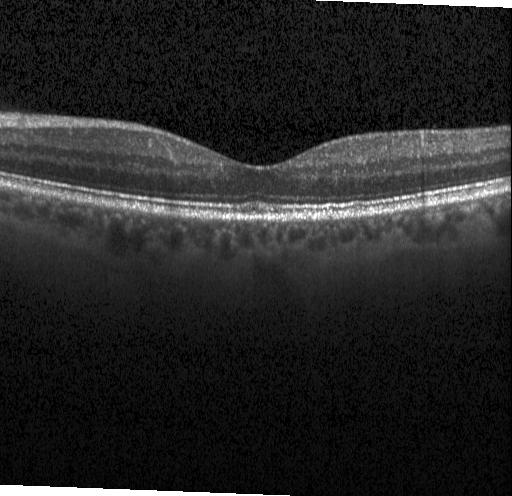
OCT line scan — OCT finding: no evidence of choroidal neovascularization, diabetic macular edema, or drusen.